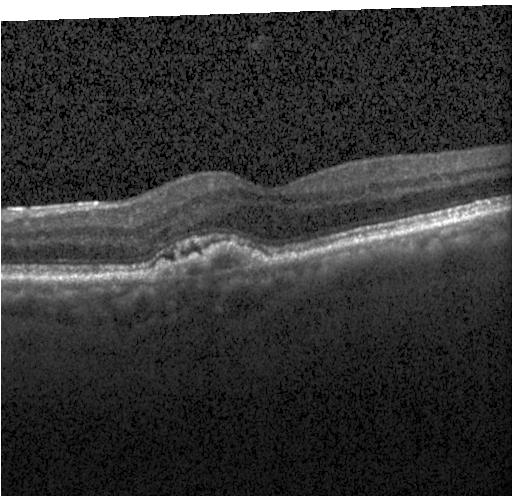

Macular OCT: a choroidal neovascular membrane.